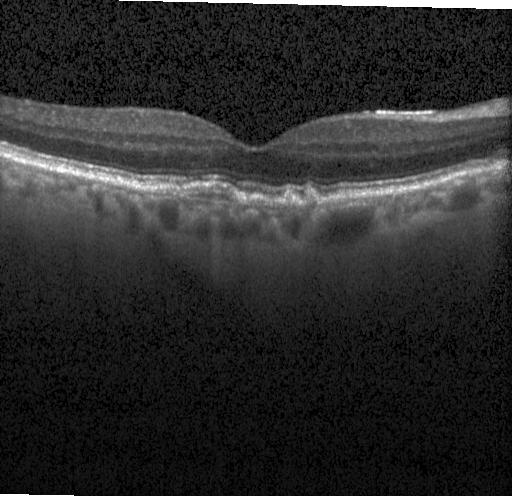

Heidelberg Spectralis OCT system. Retinal OCT cross-section.
Macular OCT: drusen.